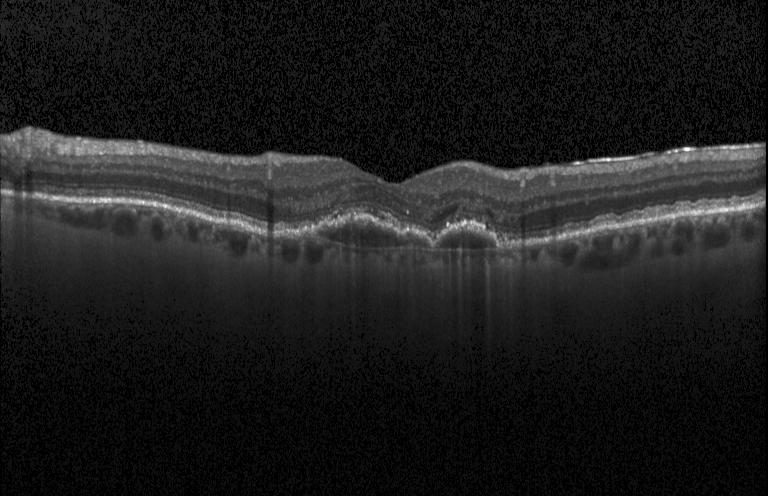

Macular scan · spectral-domain optical coherence tomography · instrument: Heidelberg Spectralis · OCT B-scan. Diagnosis: choroidal neovascularization.